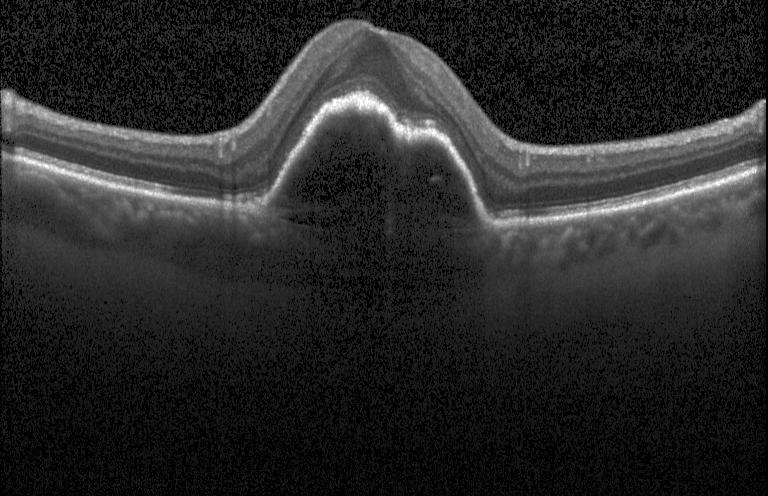
Retinal OCT cross-section · instrument: Heidelberg Spectralis.
Impression: a choroidal neovascular membrane.